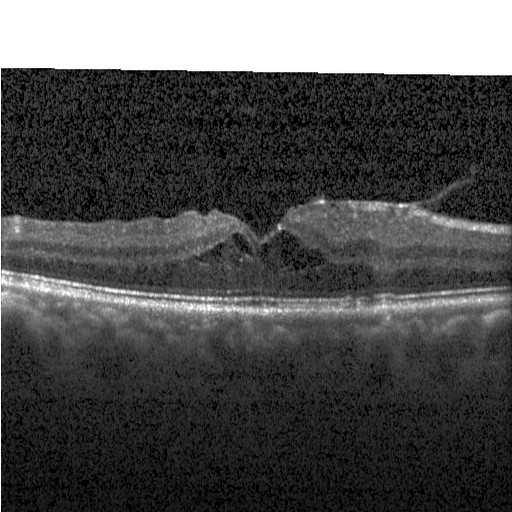
OCT line scan. Diagnosis: DME.